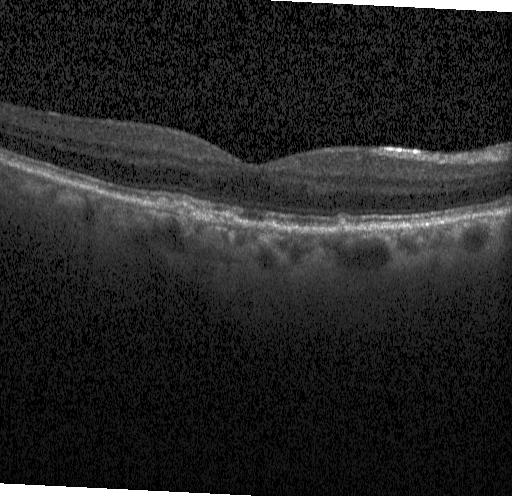
Heidelberg Spectralis; retinal OCT cross-section. Diagnosis: multiple drusen.